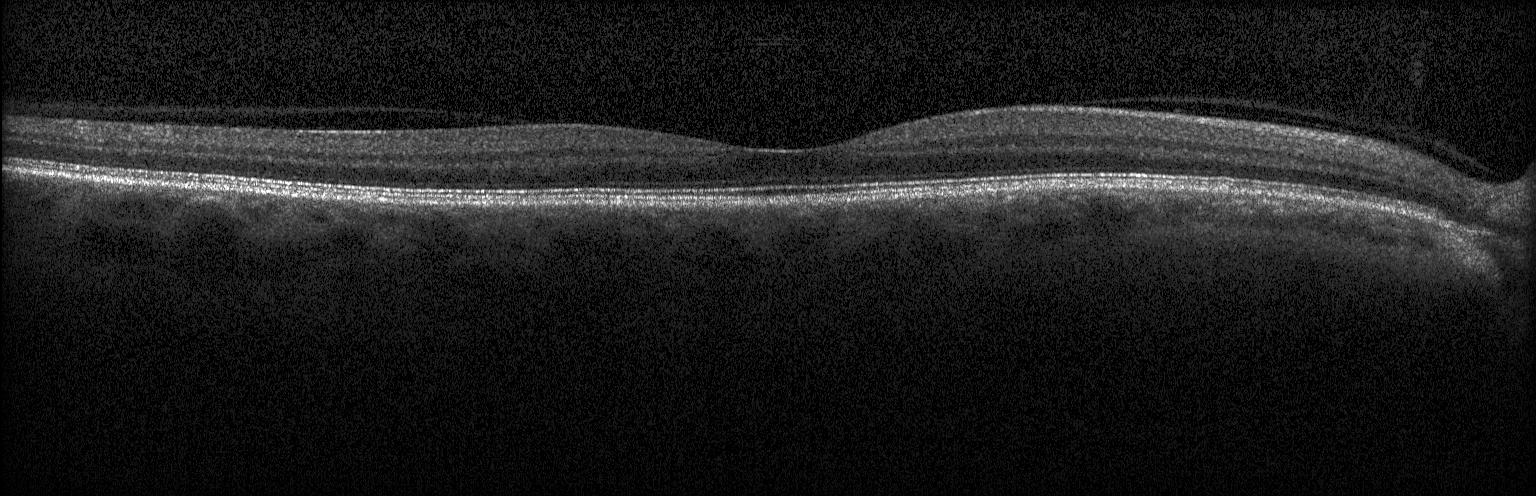

OCT B-scan showing no choroidal neovascularization, no diabetic macular edema, and no drusen.